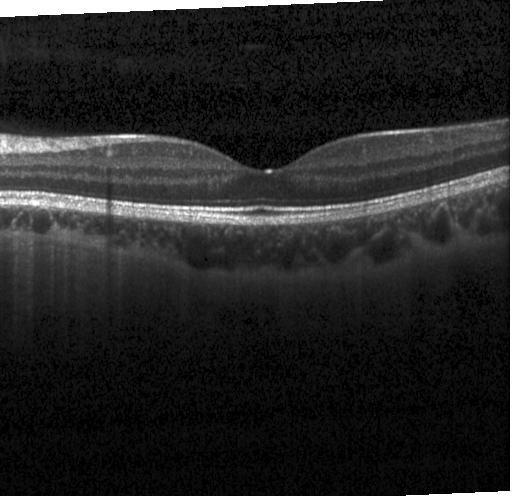

Optical coherence tomography scan
This B-scan demonstrates no choroidal neovascularization, no diabetic macular edema, and no drusen.